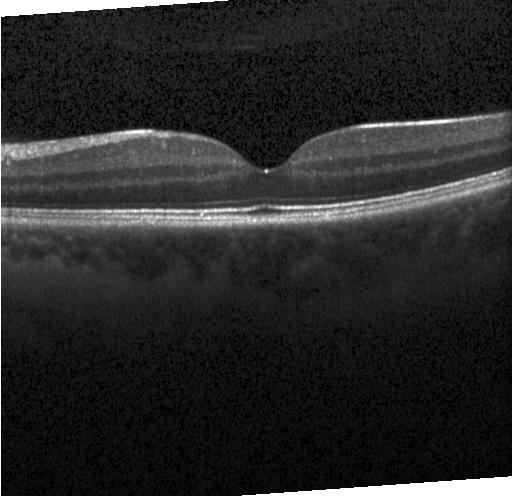

Optical coherence tomography scan · centered on the fovea · SD-OCT.
Assessment: no choroidal neovascularization, diabetic macular edema, or drusen.